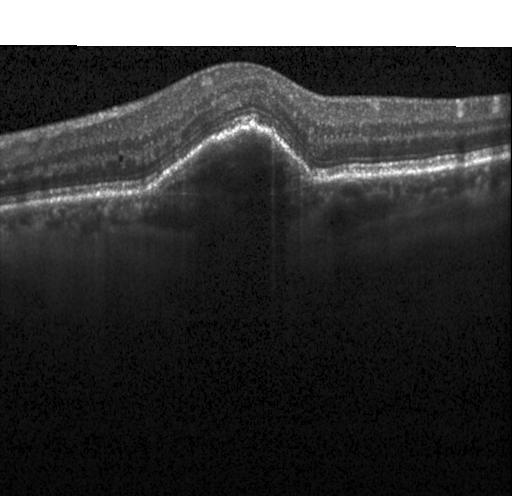
Spectral-domain OCT. Retinal OCT cross-section.
Diagnosis: a choroidal neovascular membrane.